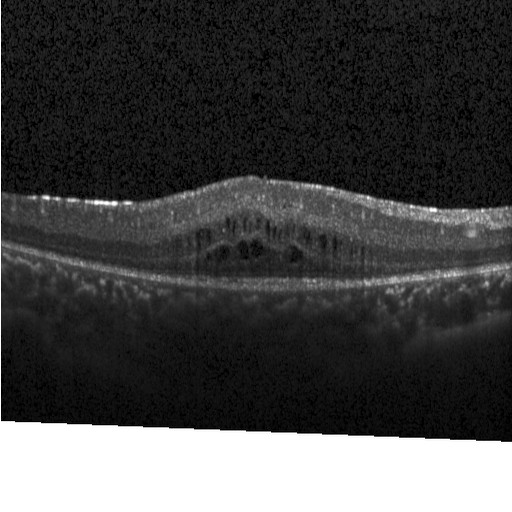
Centered on the fovea · retinal OCT B-scan. Macular OCT: DME.